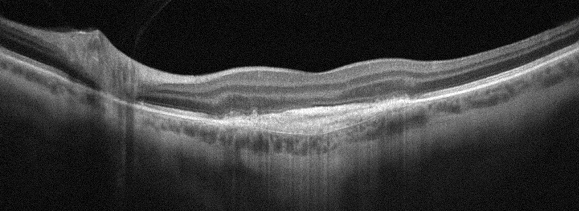
Retinal OCT B-scan, instrument: Optovue Avanti RTVue XR, through the macula, oculus sinister — The scan shows AMD.